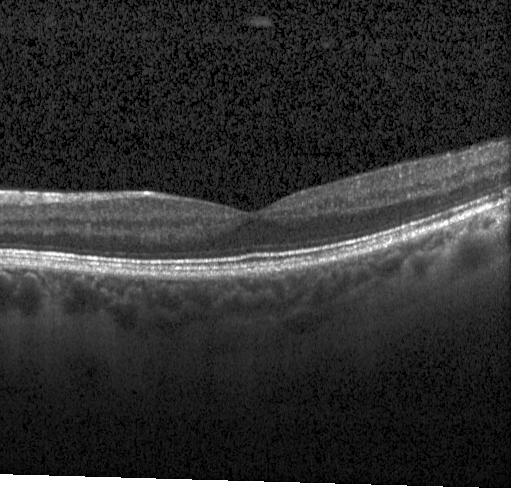
Diagnosis: no evidence of choroidal neovascularization, diabetic macular edema, or drusen.